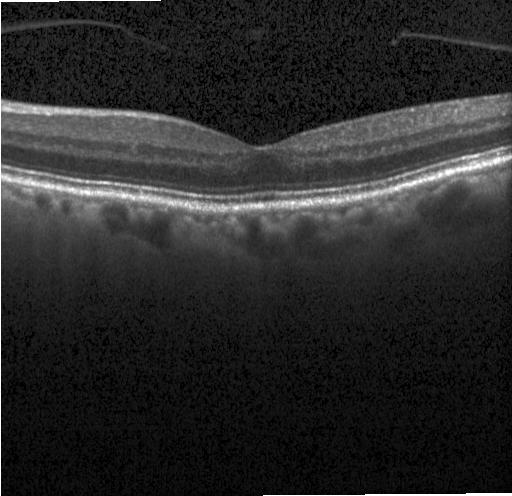

SD-OCT; instrument: Heidelberg Spectralis; optical coherence tomography scan; macular scan
Diagnosis: no choroidal neovascularization, diabetic macular edema, or drusen.